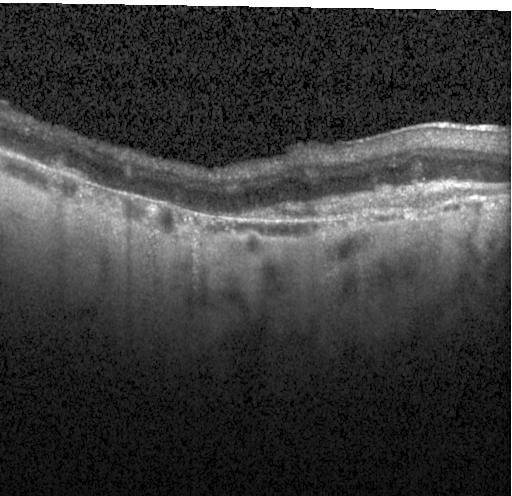

Spectral-domain optical coherence tomography, macular scan, acquired on a Heidelberg Spectralis, optical coherence tomography scan.
Dx: CNV.